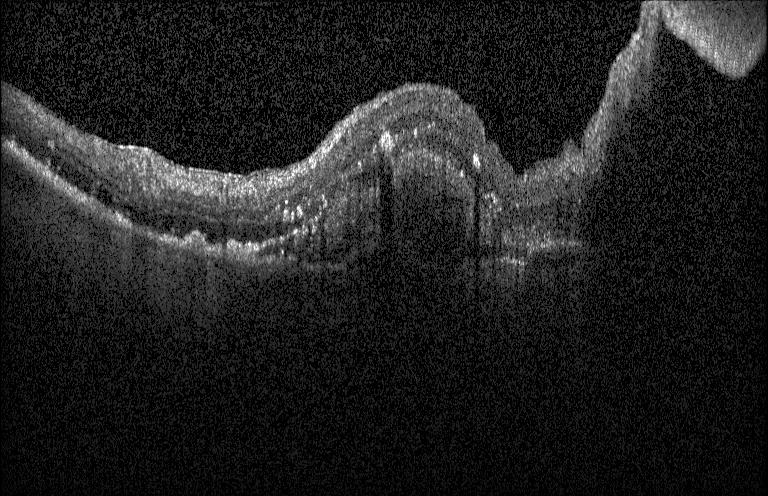
Fovea-centered · optical coherence tomography scan
Assessment: choroidal neovascularization (CNV).